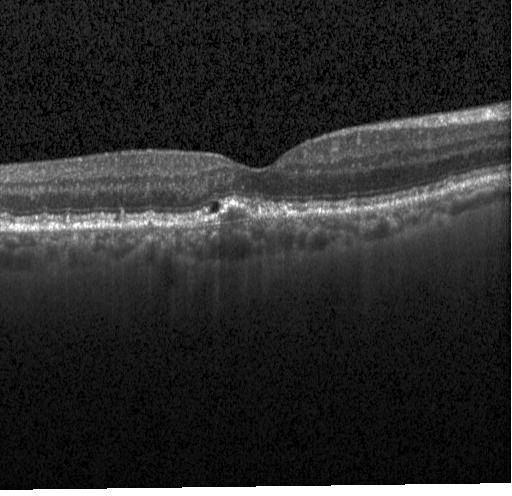
Macular OCT demonstrating choroidal neovascularization.